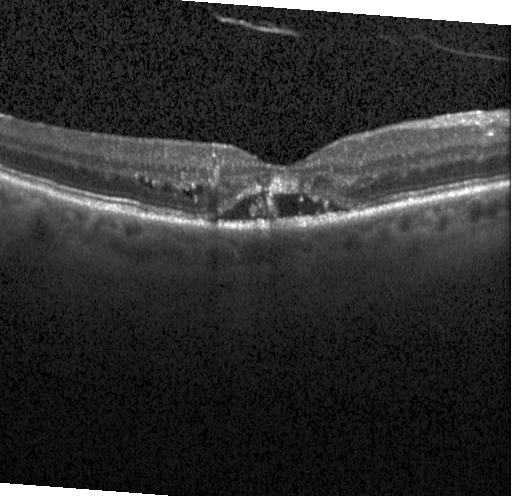
Optical coherence tomography B-scan — Impression: choroidal neovascularization.